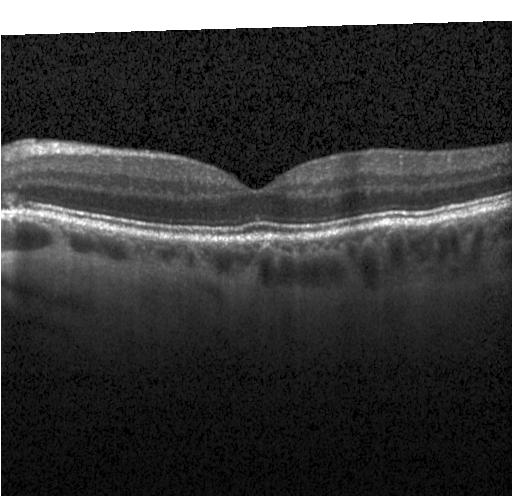

Instrument: Heidelberg Spectralis. Optical coherence tomography B-scan. Fovea-centered. Assessment: neither CNV, DME, nor drusen.